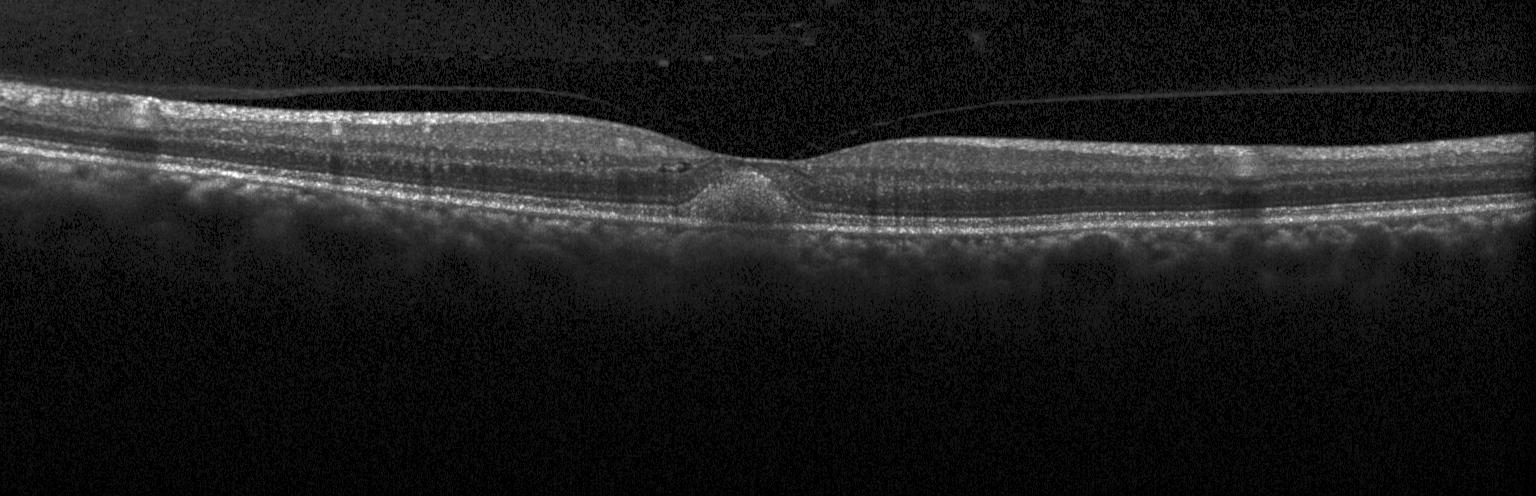

Optical coherence tomography B-scan — Diagnosis: a choroidal neovascular membrane.